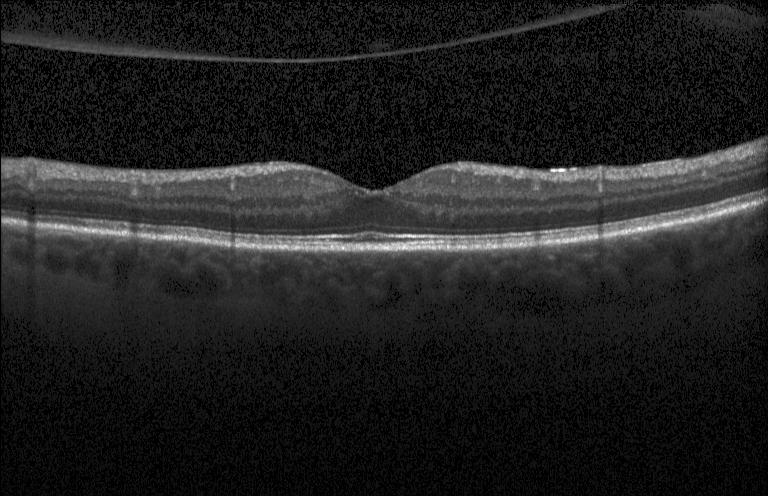
Retinal OCT B-scan, fovea-centered, SD-OCT, Heidelberg Spectralis OCT system
Impression: neither choroidal neovascularization, diabetic macular edema, nor drusen.